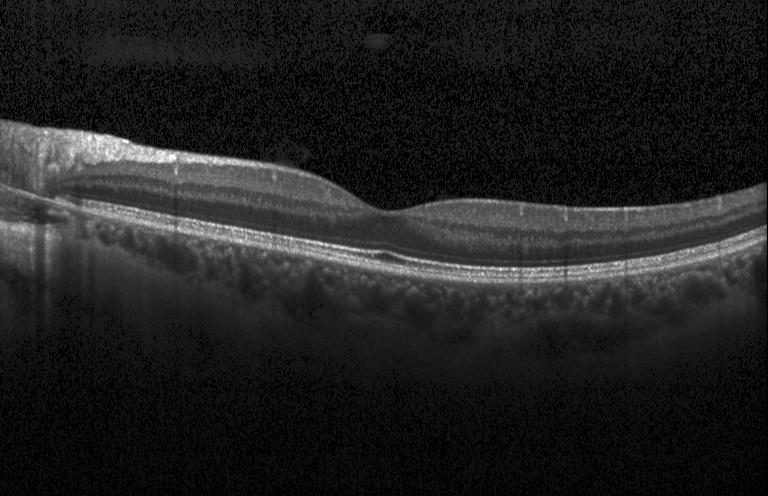 Horizontal scan through the fovea; SD-OCT; OCT line scan
Macular OCT: neither choroidal neovascularization, diabetic macular edema, nor drusen.